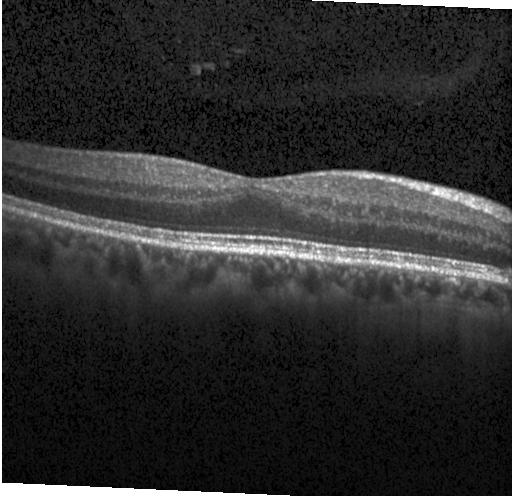
Optical coherence tomography B-scan; spectral-domain optical coherence tomography.
This B-scan demonstrates no choroidal neovascularization, no diabetic macular edema, and no drusen.